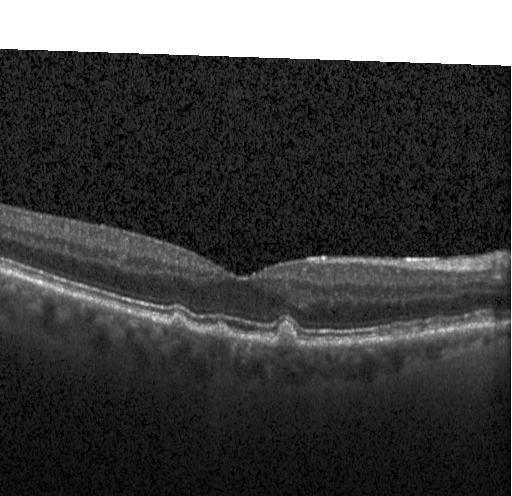

Macular OCT demonstrating drusen.